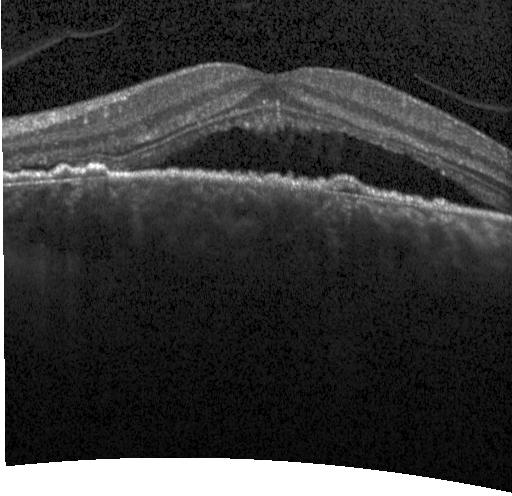

Impression: a choroidal neovascular membrane.